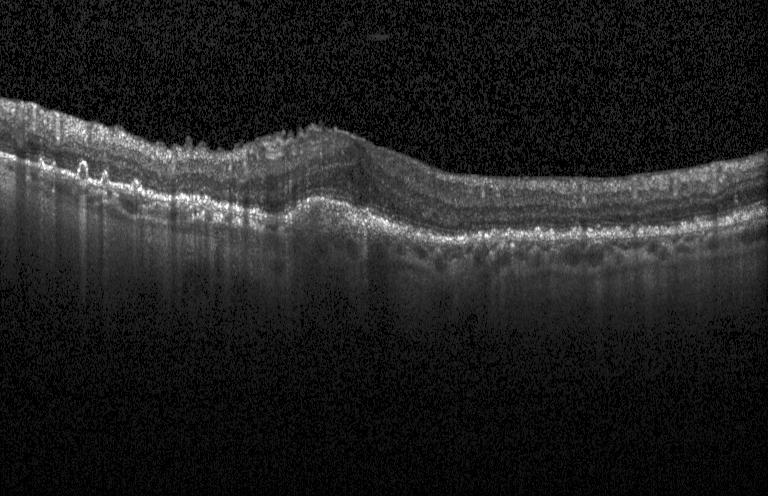
Assessment: choroidal neovascularization (CNV).